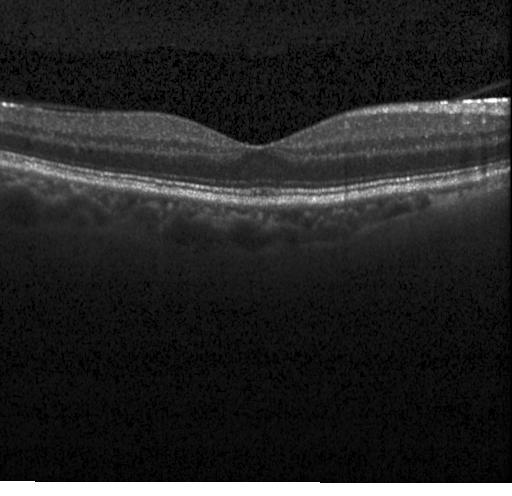 SD-OCT · optical coherence tomography B-scan · centered on the fovea — Impression: no CNV, DME, or drusen.